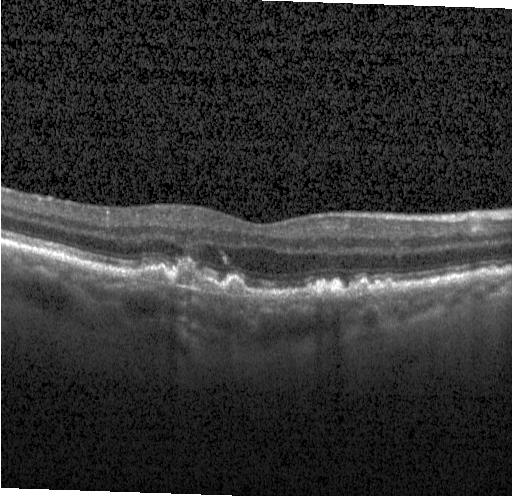
Macular OCT: multiple drusen.